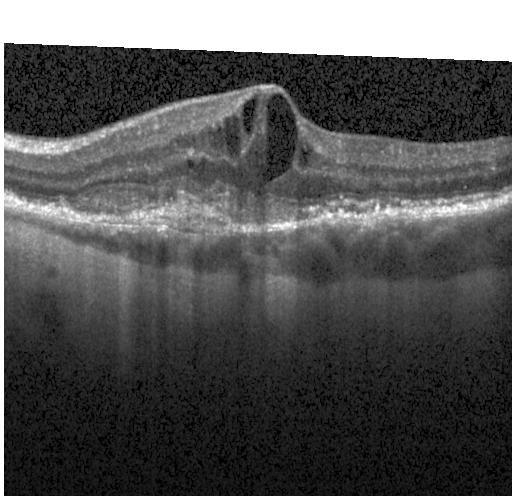
Macular OCT demonstrating a choroidal neovascular membrane.